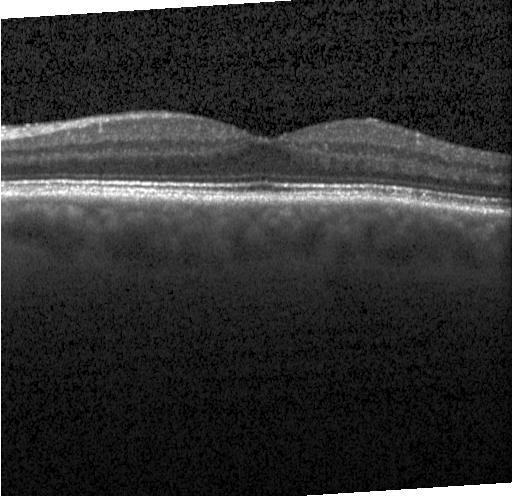 Dx: neither choroidal neovascularization, diabetic macular edema, nor drusen.